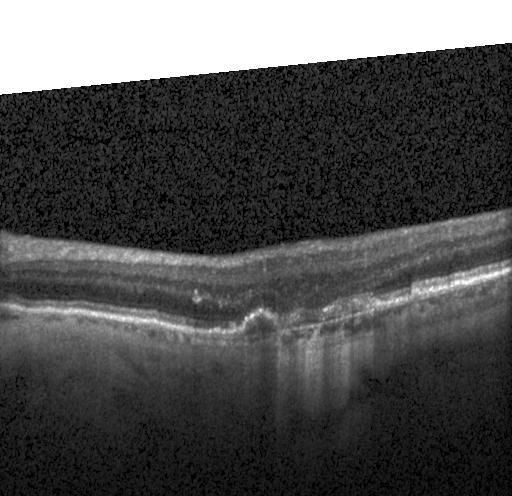
Finding: a choroidal neovascular membrane.